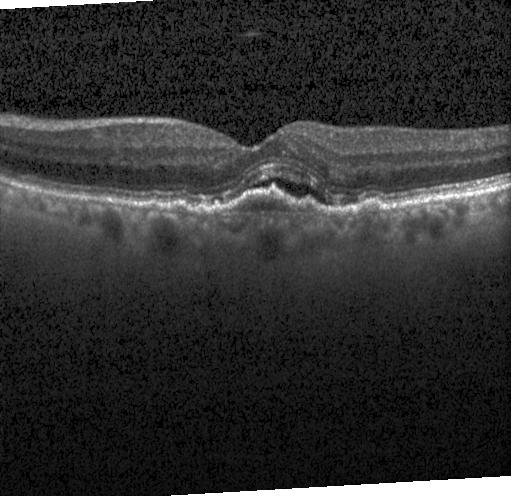 Optical coherence tomography B-scan, horizontal scan through the fovea, SD-OCT
Impression: choroidal neovascularization.